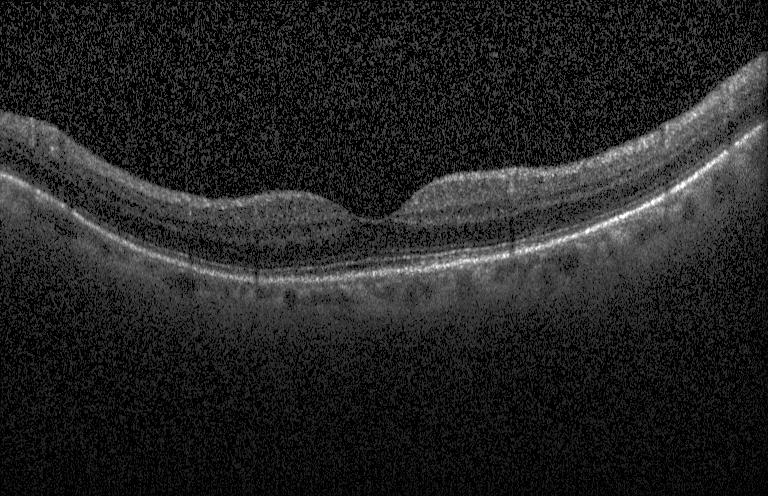
Retinal OCT cross-section — Finding: no choroidal neovascularization, no diabetic macular edema, and no drusen.